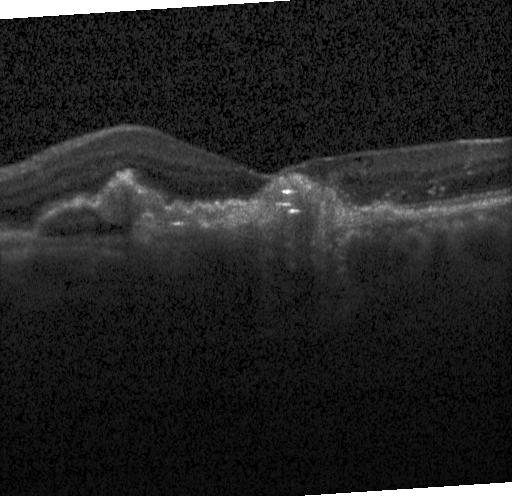
OCT scan showing a choroidal neovascular membrane.